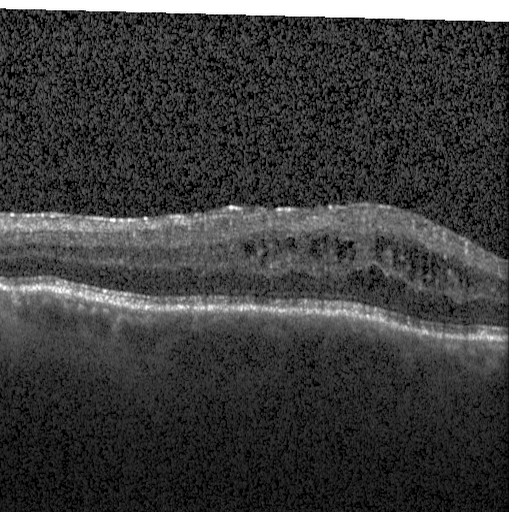 Macular OCT demonstrating diabetic macular edema (DME).